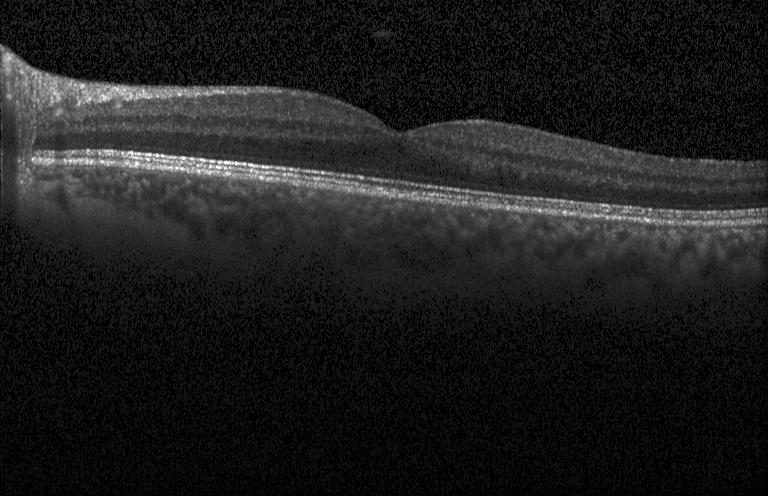

Spectral-domain optical coherence tomography, retinal OCT cross-section, Heidelberg Spectralis OCT system, horizontal scan through the fovea. Macular OCT: neither choroidal neovascularization, diabetic macular edema, nor drusen.